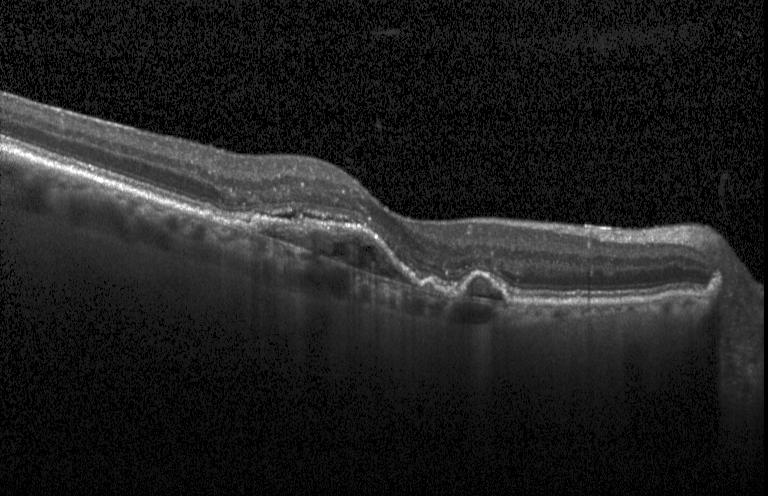

OCT line scan — Macular OCT: a choroidal neovascular membrane.